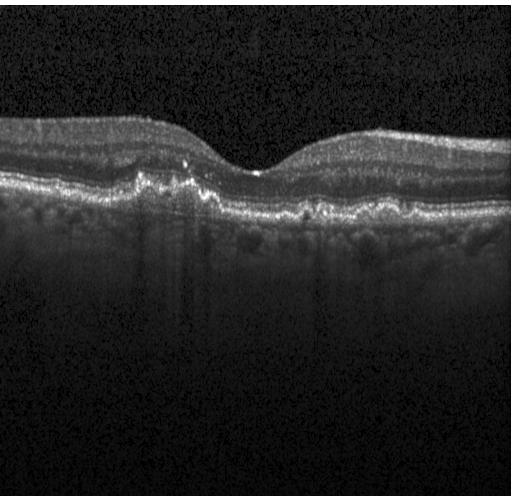
OCT B-scan; acquired on a Heidelberg Spectralis
Diagnosis: choroidal neovascularization (CNV).